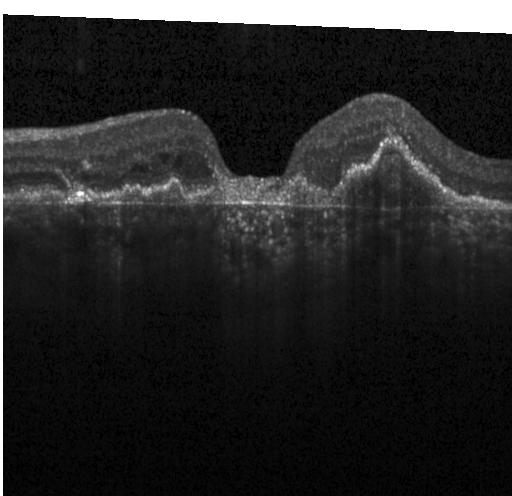
OCT line scan · spectral-domain OCT · centered on the fovea.
Assessment: choroidal neovascularization (CNV).